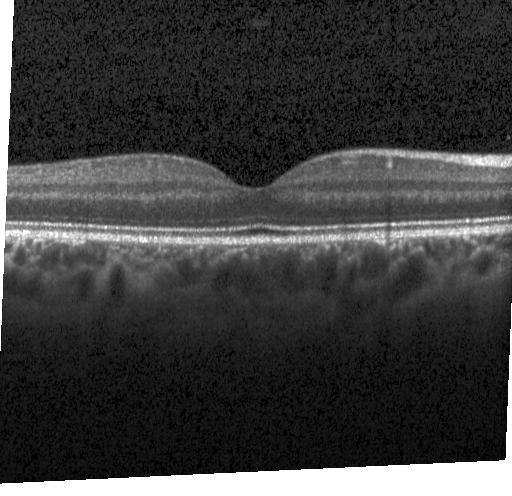

Optical coherence tomography scan, spectral-domain optical coherence tomography, through the macula, Heidelberg Spectralis OCT system — Impression: no evidence of CNV, DME, or drusen.